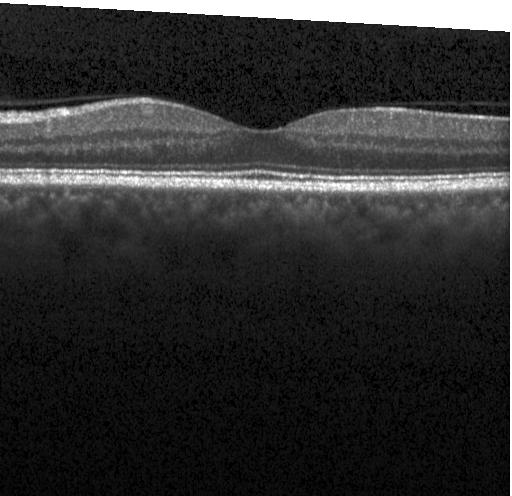

Heidelberg Spectralis OCT system. Spectral-domain OCT. Retinal OCT cross-section
Diagnosis: no choroidal neovascularization, no diabetic macular edema, and no drusen.